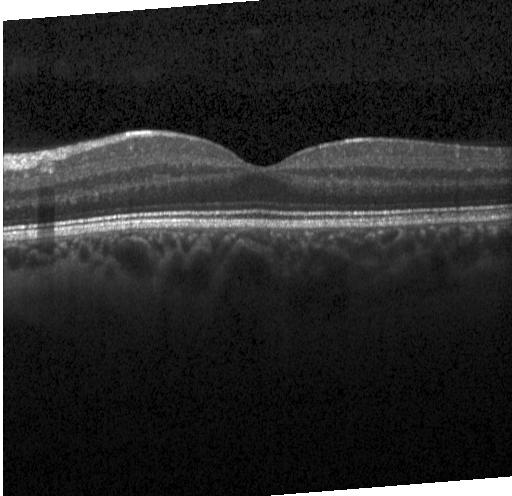
Macular OCT demonstrating neither CNV, DME, nor drusen.